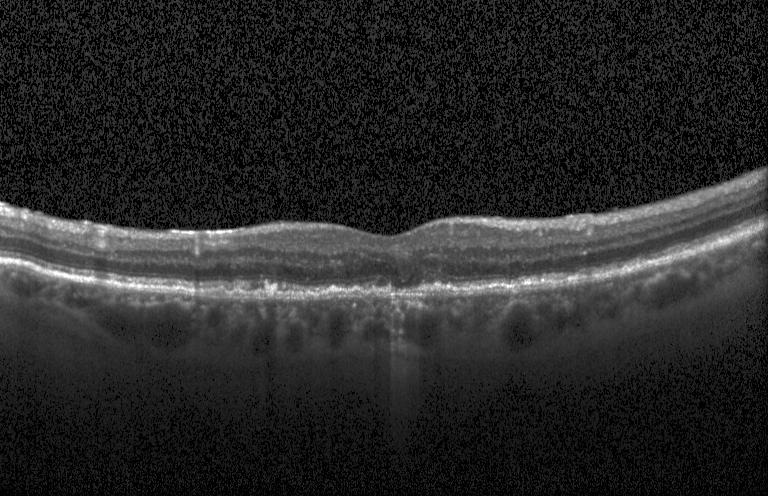

Macular OCT demonstrating a choroidal neovascular membrane.